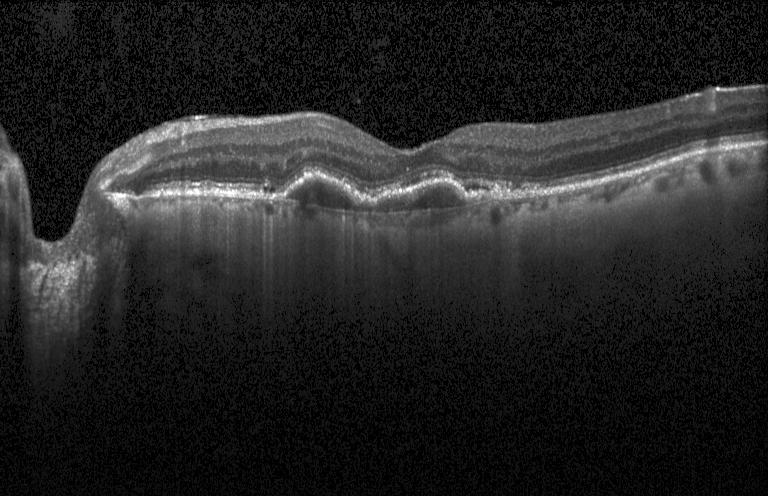

OCT line scan. Spectral-domain OCT — OCT finding: a choroidal neovascular membrane.